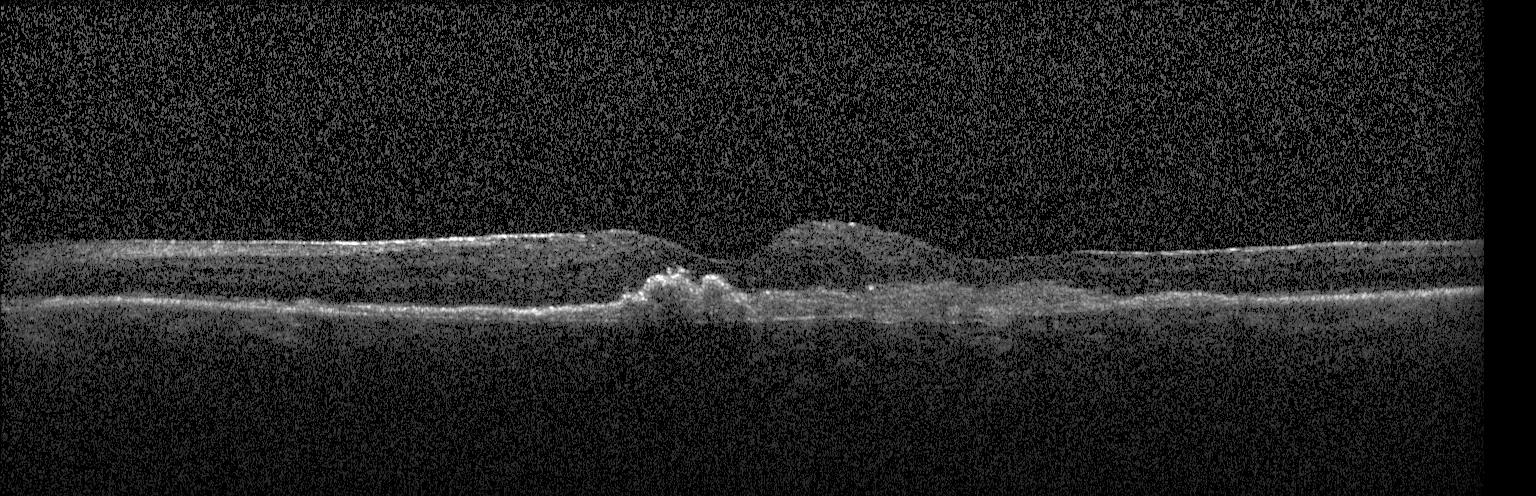 Retinal OCT cross-section. Horizontal scan through the fovea — Assessment: a choroidal neovascular membrane.